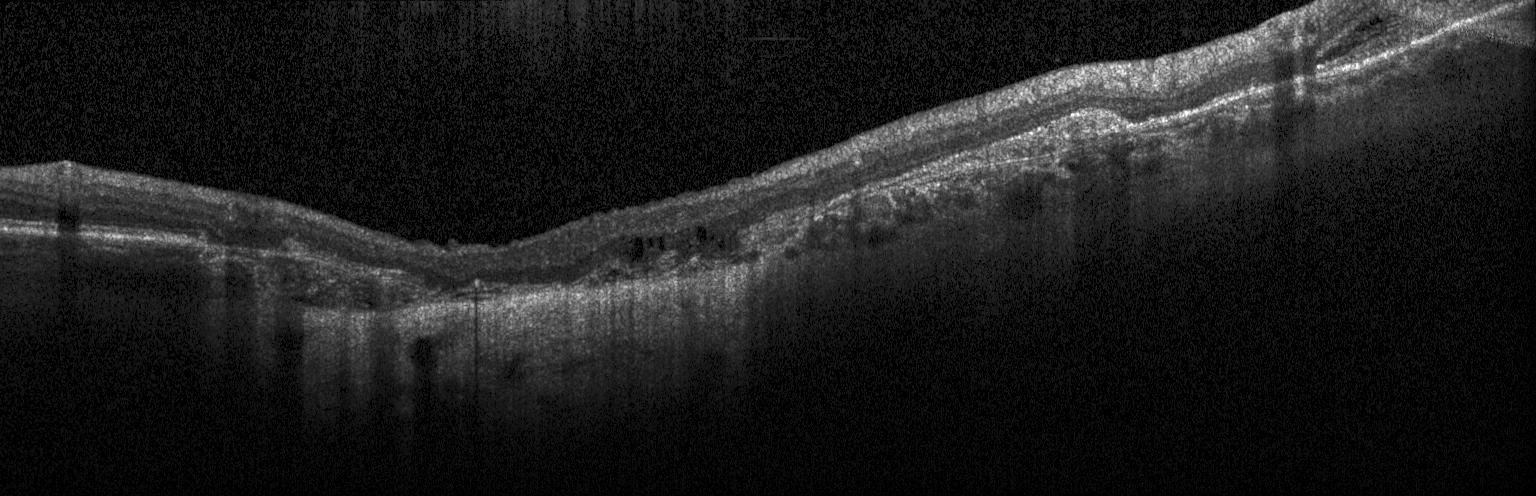 SD-OCT · acquired on a Heidelberg Spectralis · OCT line scan · through the macula — This B-scan demonstrates choroidal neovascularization.